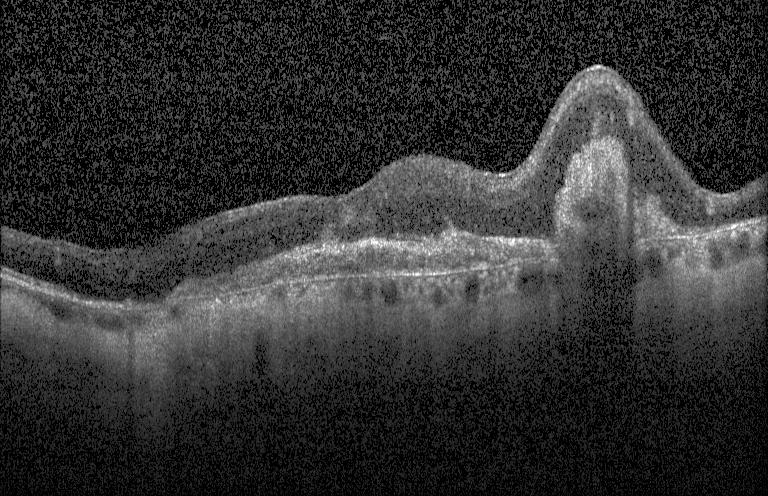
Heidelberg Spectralis OCT system; spectral-domain optical coherence tomography; optical coherence tomography scan
Impression: a choroidal neovascular membrane.